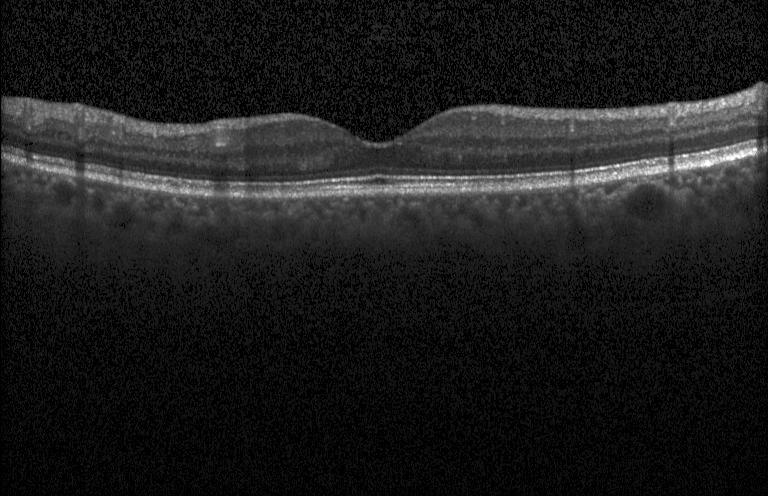 SD-OCT; OCT B-scan; macular scan; instrument: Heidelberg Spectralis.
Impression: no CNV, DME, or drusen.